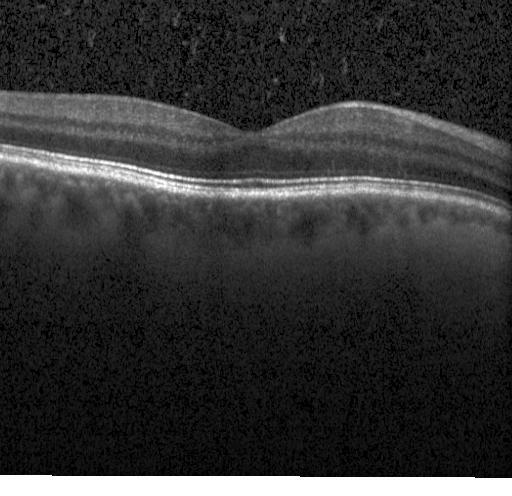
Retinal OCT B-scan — Diagnosis: neither CNV, DME, nor drusen.